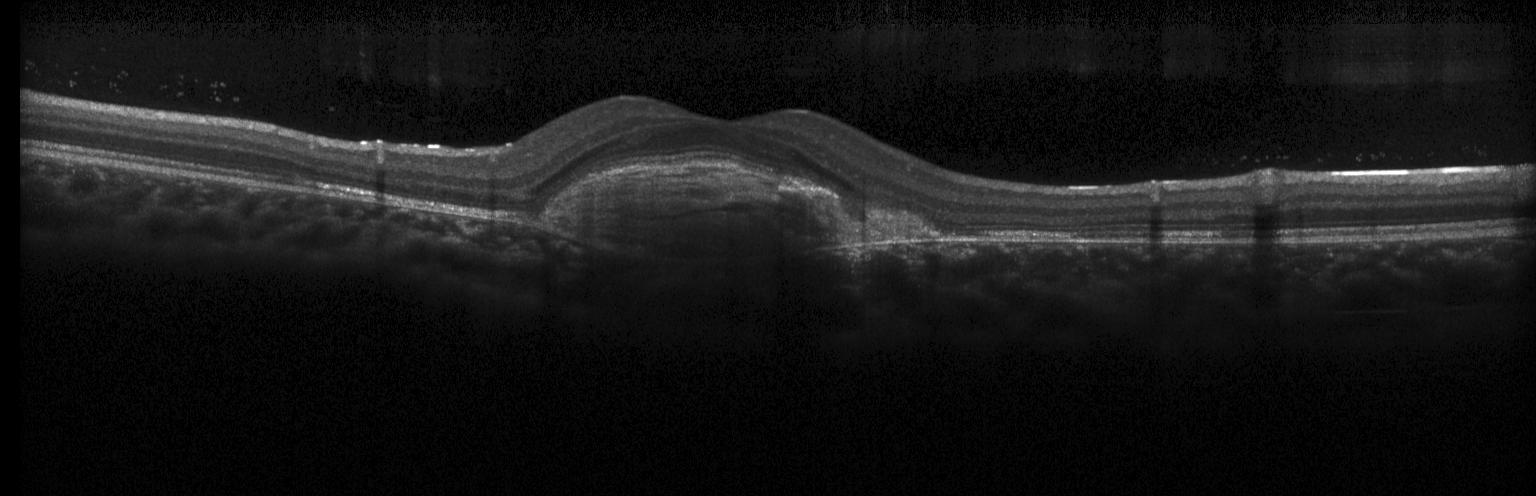
Diagnosis: a choroidal neovascular membrane.